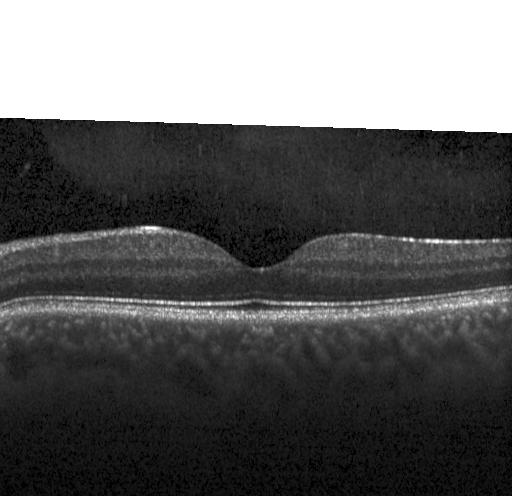 Centered on the fovea. Optical coherence tomography scan.
Impression: no choroidal neovascularization, no diabetic macular edema, and no drusen.